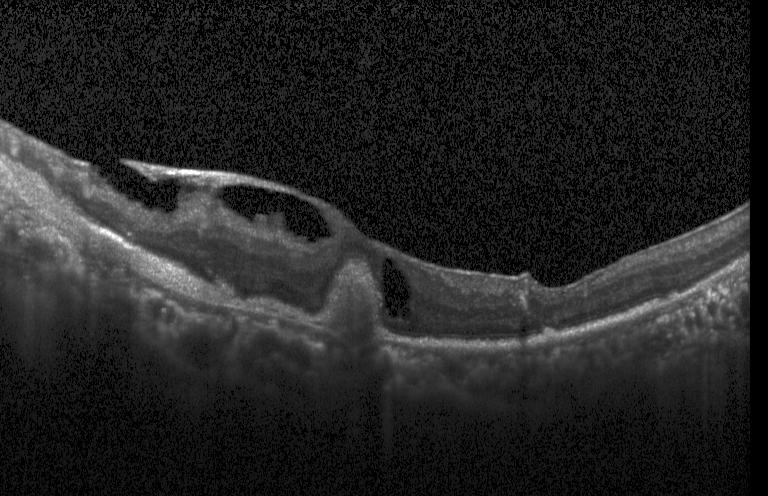 Retinal OCT B-scan. Spectral-domain optical coherence tomography. Fovea-centered
This B-scan demonstrates a choroidal neovascular membrane.